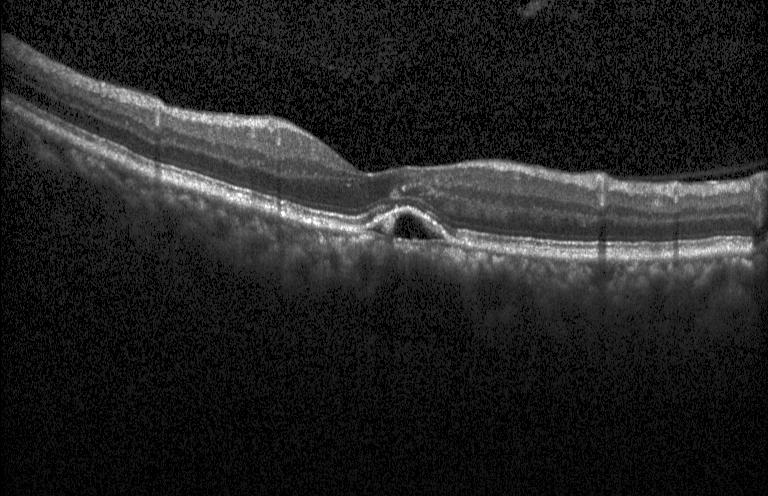

This B-scan demonstrates CNV.